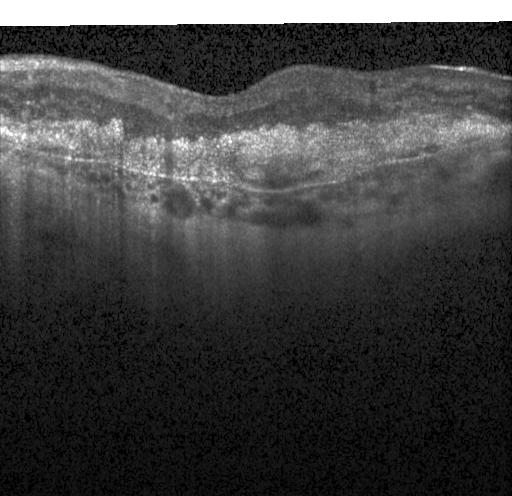 Optical coherence tomography scan
Macular OCT: choroidal neovascularization.